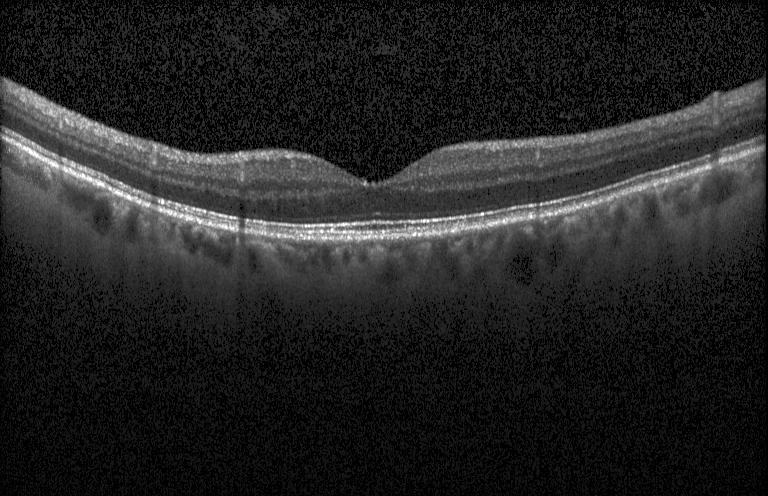
Assessment: no CNV, DME, or drusen.